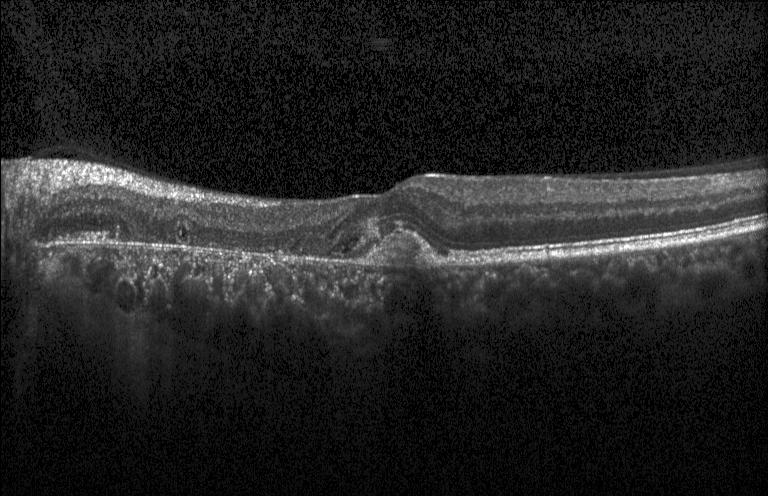 Macular OCT demonstrating a choroidal neovascular membrane.